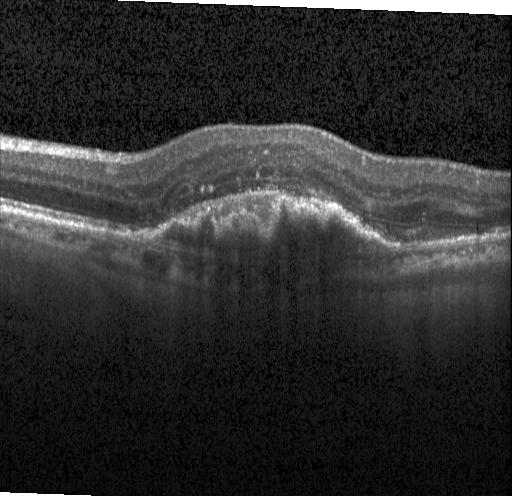

Retinal OCT B-scan. Macular OCT: a choroidal neovascular membrane.